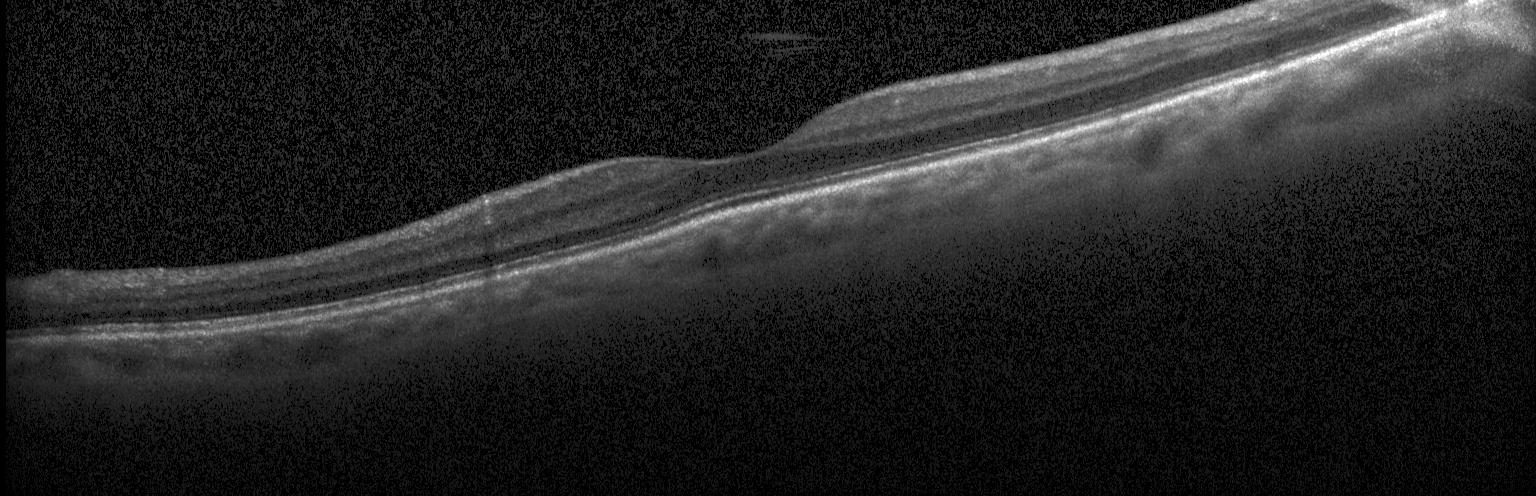

Spectral-domain optical coherence tomography. Retinal OCT cross-section. Heidelberg Spectralis. Assessment: no choroidal neovascularization, diabetic macular edema, or drusen.